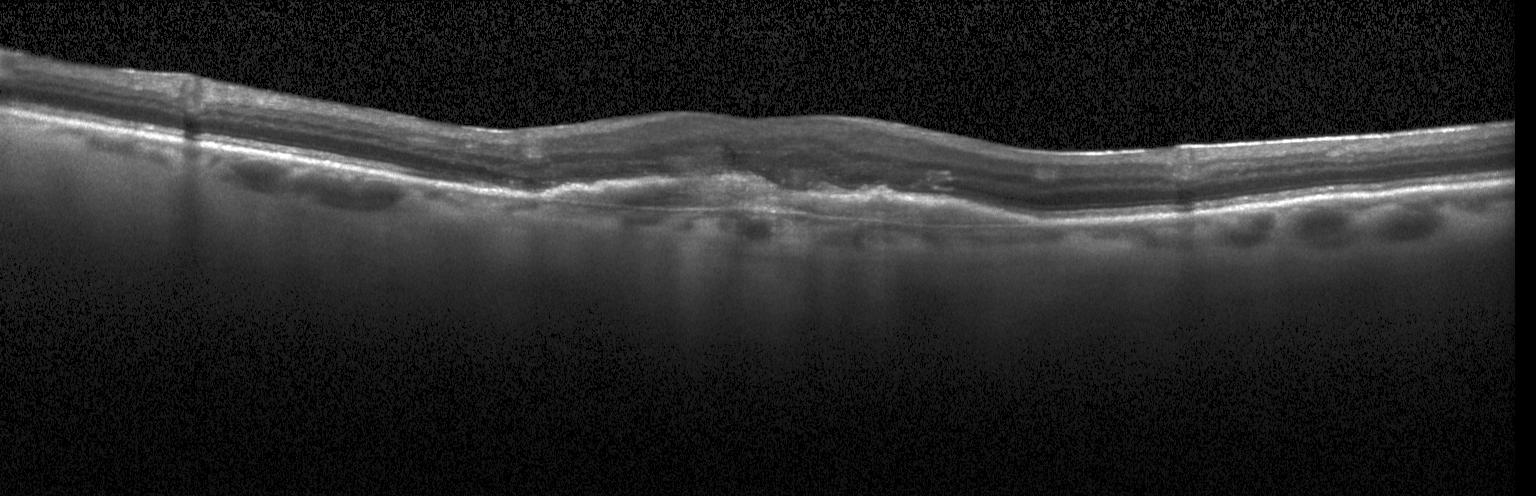

Optical coherence tomography B-scan — Diagnosis: CNV.